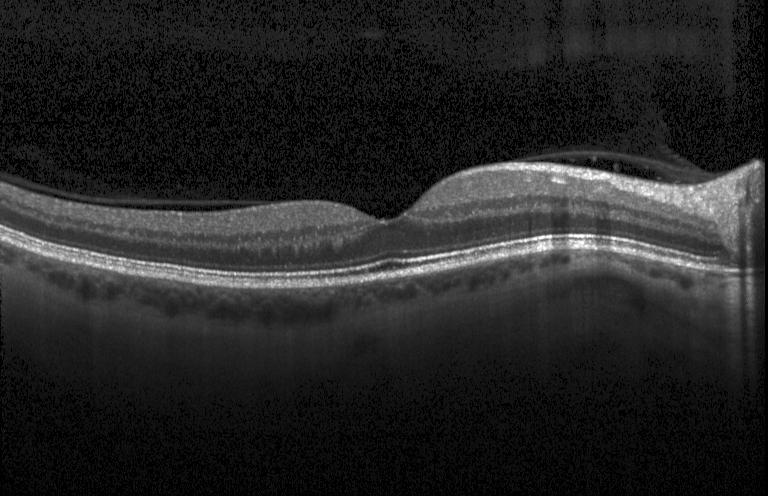

Fovea-centered; OCT line scan; instrument: Heidelberg Spectralis. Impression: no evidence of CNV, DME, or drusen.